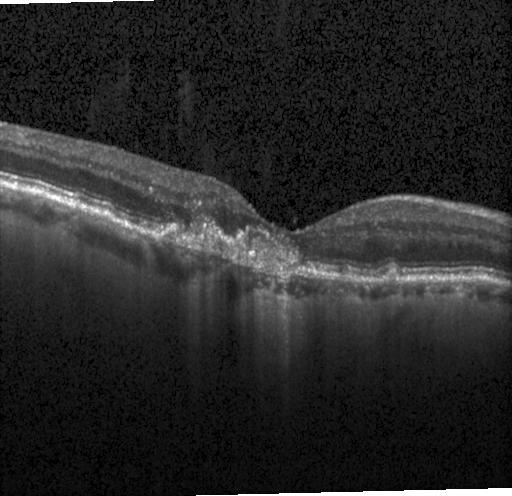
OCT B-scan. Spectral-domain optical coherence tomography
Diagnosis: choroidal neovascularization (CNV).